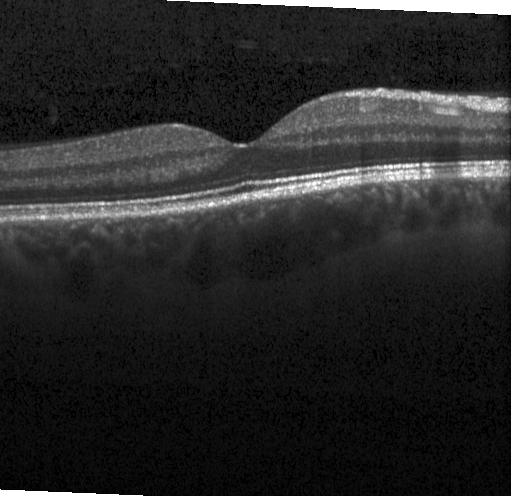
Retinal OCT B-scan. SD-OCT. Centered on the fovea — Diagnosis: no CNV, DME, or drusen.